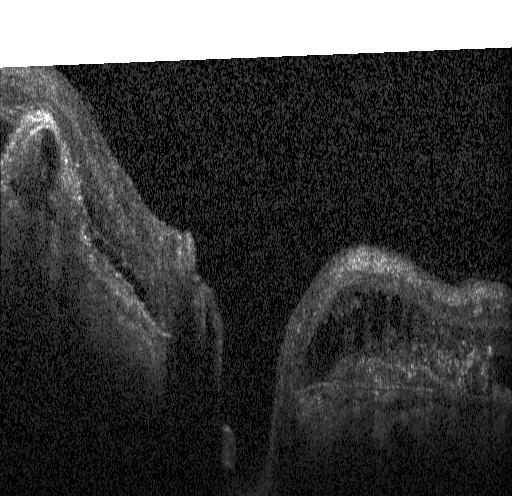
Diagnosis: choroidal neovascularization (CNV).